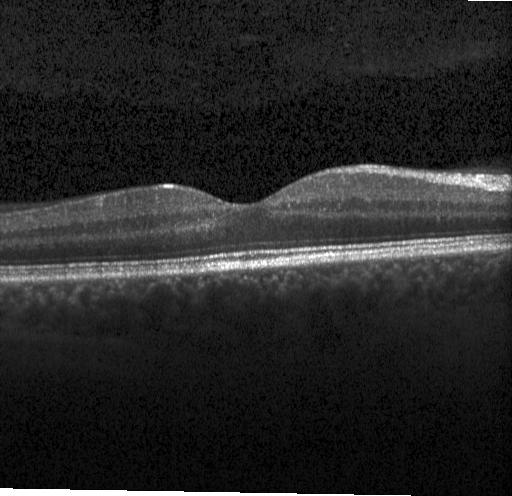
Heidelberg Spectralis, through the macula, spectral-domain optical coherence tomography, optical coherence tomography scan. Diagnosis: neither choroidal neovascularization, diabetic macular edema, nor drusen.